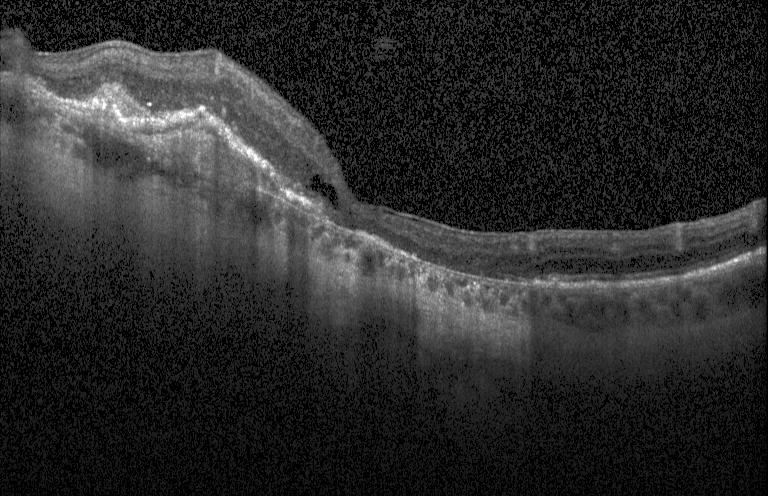

OCT finding: a choroidal neovascular membrane.